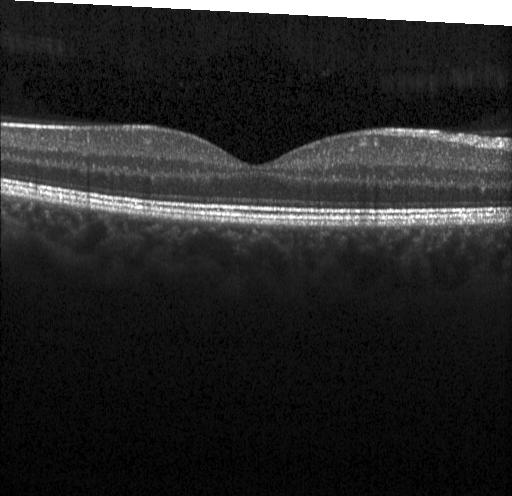

Impression: no CNV, no DME, and no drusen.